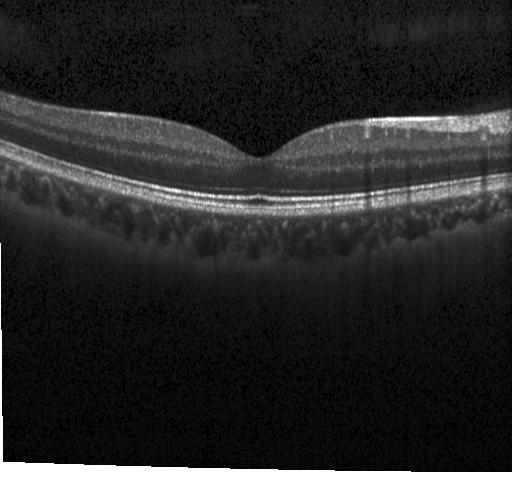

Instrument: Heidelberg Spectralis, spectral-domain OCT, retinal OCT cross-section, horizontal scan through the fovea — Macular OCT: no choroidal neovascularization, no diabetic macular edema, and no drusen.